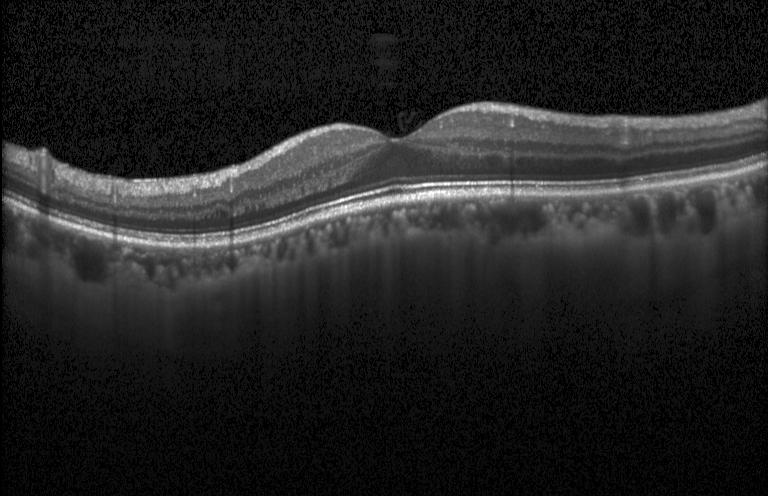
Finding: neither choroidal neovascularization, diabetic macular edema, nor drusen.